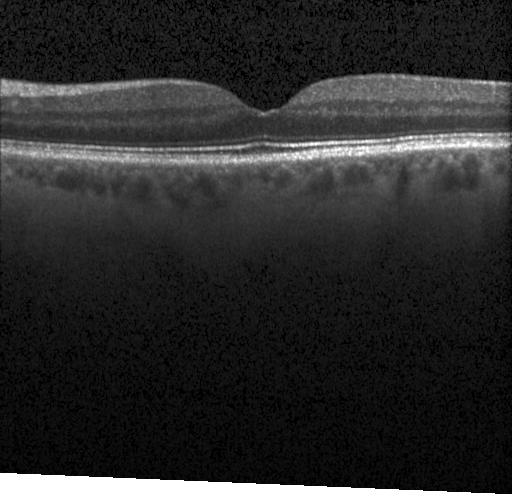
Diagnosis: no choroidal neovascularization, no diabetic macular edema, and no drusen.